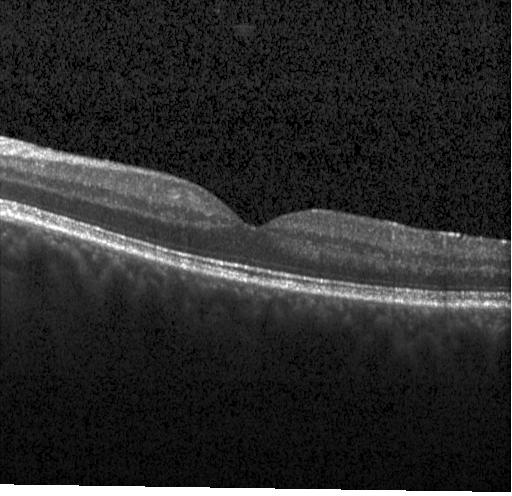
Through the macula · spectral-domain OCT · retinal OCT cross-section · Heidelberg Spectralis. Macular OCT: no evidence of choroidal neovascularization, diabetic macular edema, or drusen.